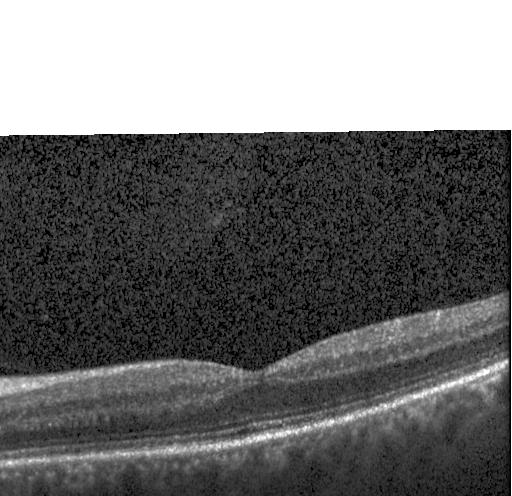

SD-OCT; Heidelberg Spectralis; macular scan; optical coherence tomography B-scan.
Macular OCT: no choroidal neovascularization, diabetic macular edema, or drusen.